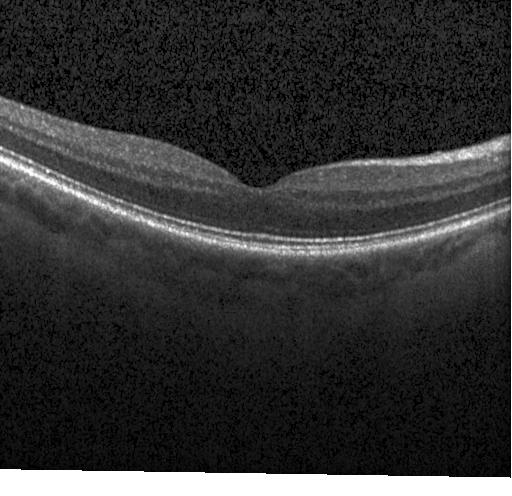 OCT line scan, instrument: Heidelberg Spectralis, fovea-centered, SD-OCT
Finding: no choroidal neovascularization, diabetic macular edema, or drusen.